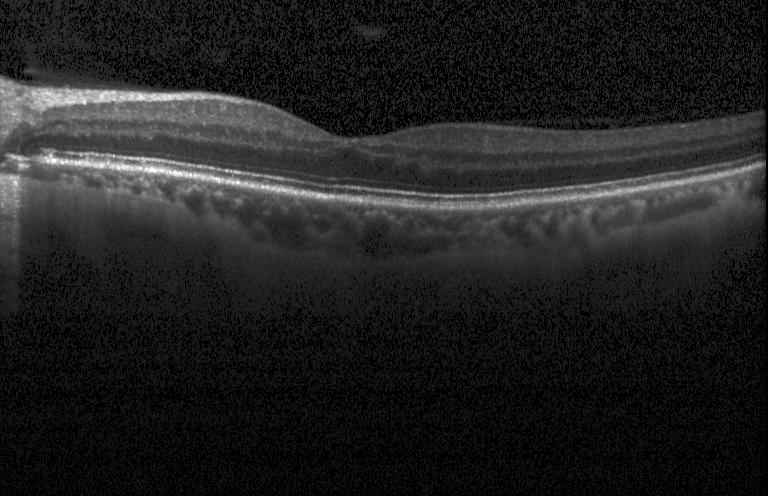

Impression: no choroidal neovascularization, diabetic macular edema, or drusen.